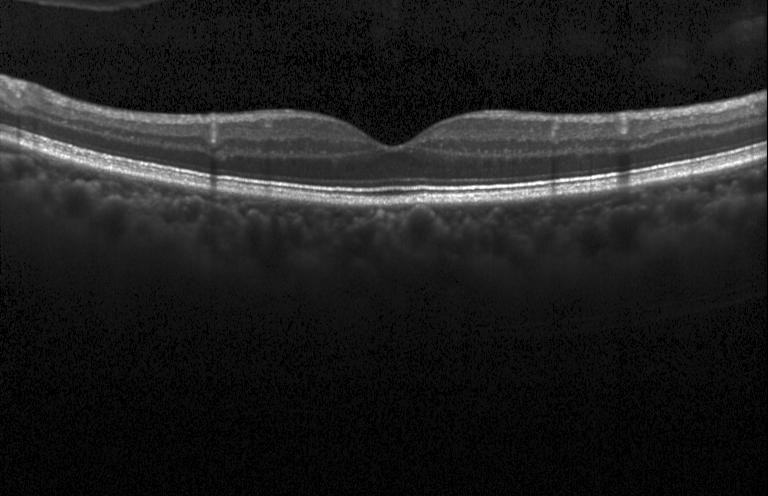

Fovea-centered · retinal OCT B-scan. This B-scan demonstrates no choroidal neovascularization, no diabetic macular edema, and no drusen.